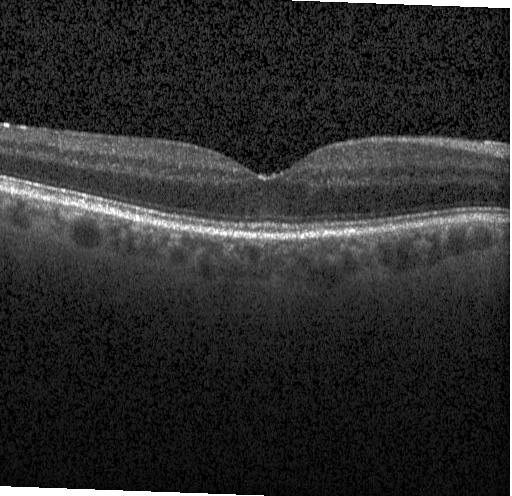

Optical coherence tomography scan — Impression: no CNV, DME, or drusen.